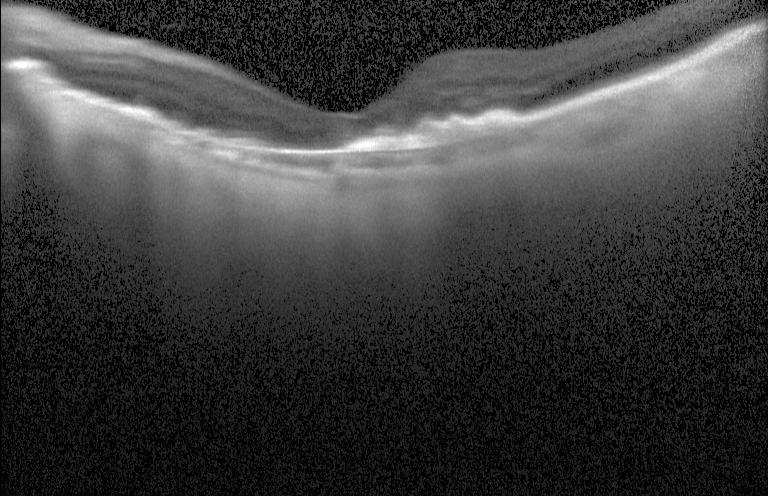

OCT finding: a choroidal neovascular membrane.